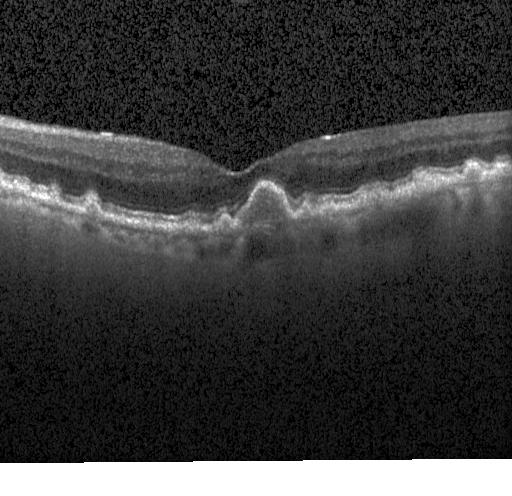 Optical coherence tomography B-scan. SD-OCT. Acquired on a Heidelberg Spectralis — Diagnosis: drusen.